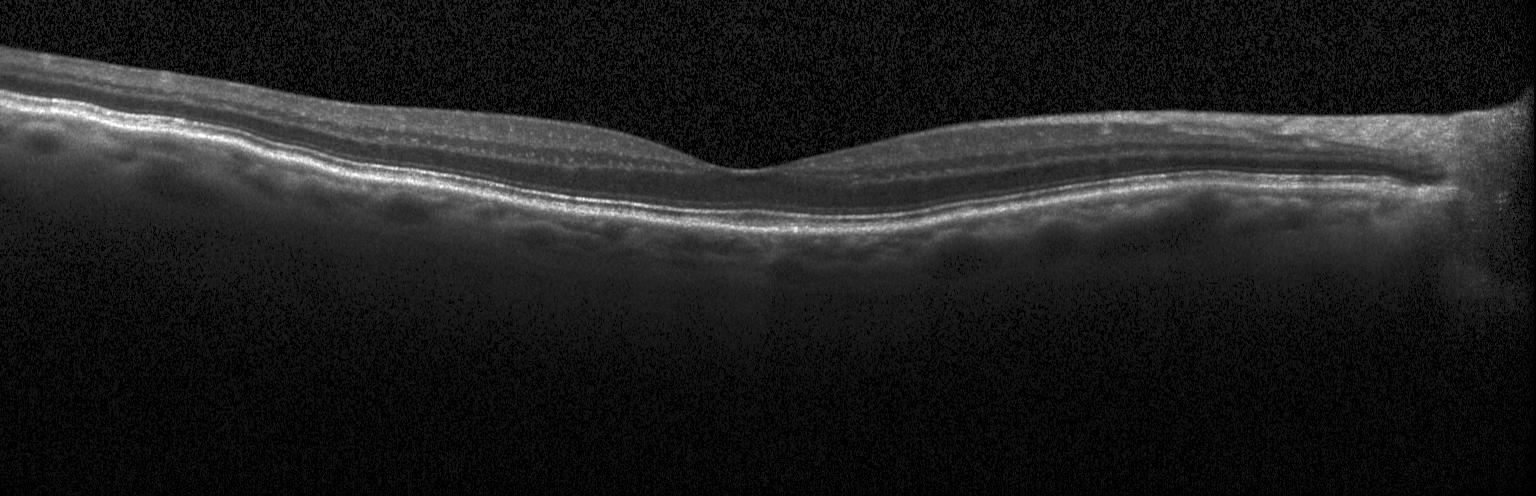
OCT scan showing no choroidal neovascularization, diabetic macular edema, or drusen.